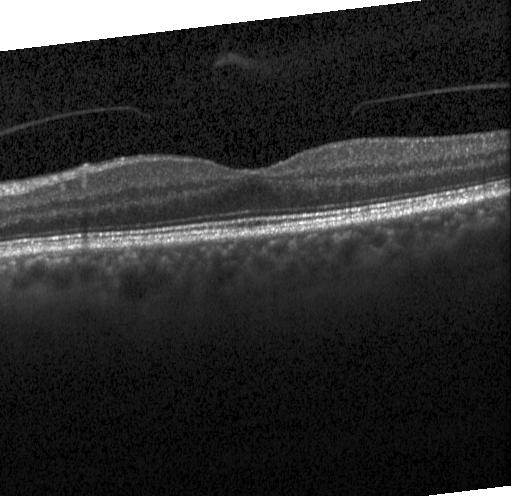 Retinal OCT B-scan. Horizontal scan through the fovea. Acquired on a Heidelberg Spectralis. SD-OCT
The scan shows no evidence of CNV, DME, or drusen.